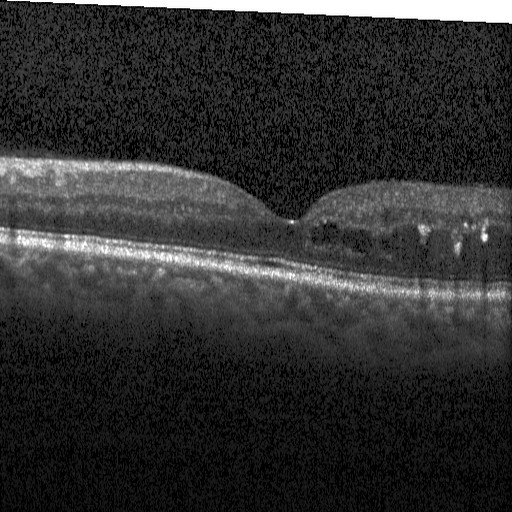
Heidelberg Spectralis OCT system, through the macula, SD-OCT, OCT line scan. This B-scan demonstrates diabetic macular edema (DME).